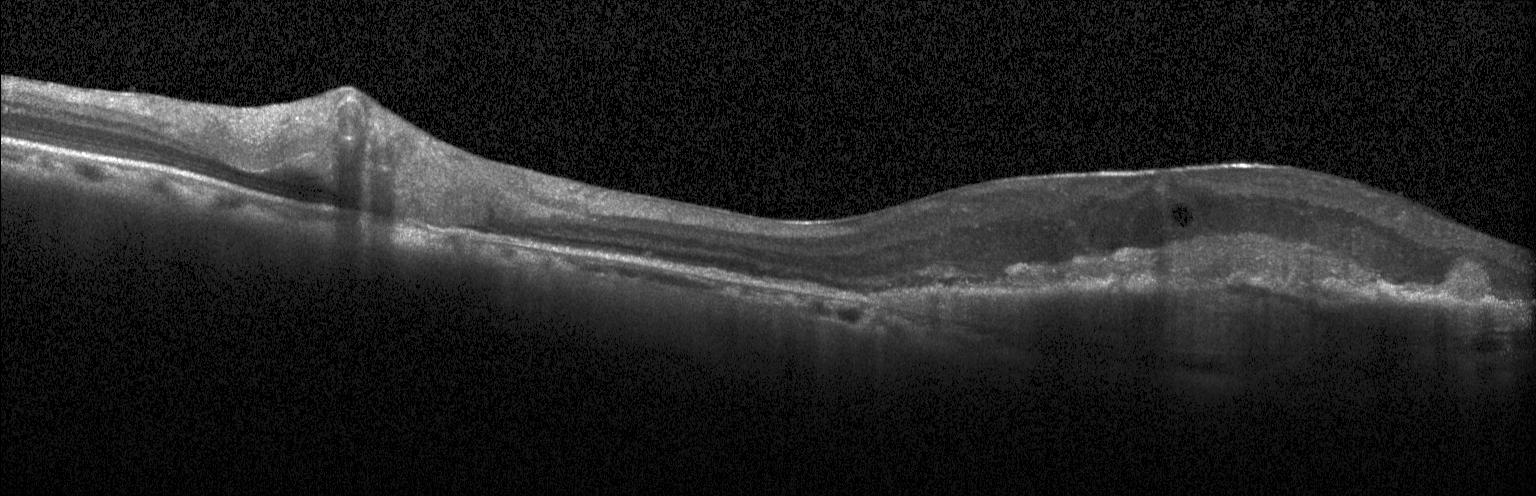 Spectral-domain OCT B-scan: a choroidal neovascular membrane.